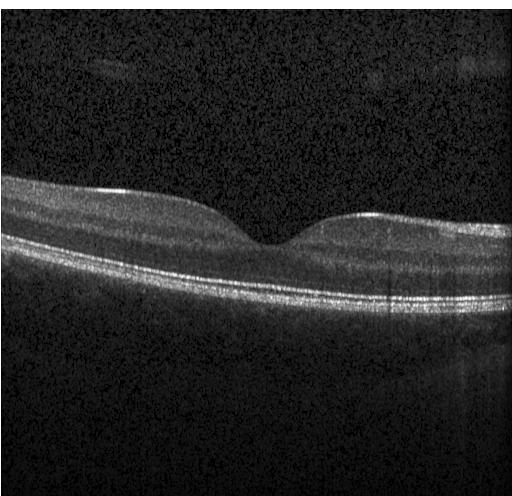

Optical coherence tomography scan. The scan shows no CNV, DME, or drusen.